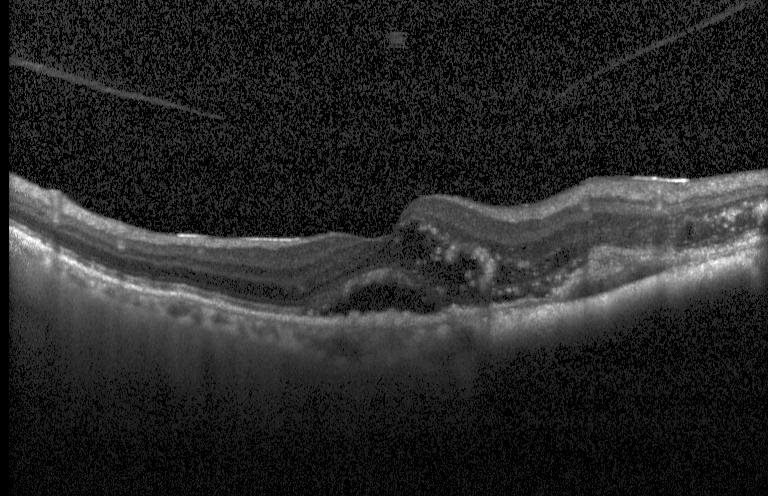

Spectral-domain OCT B-scan: choroidal neovascularization.